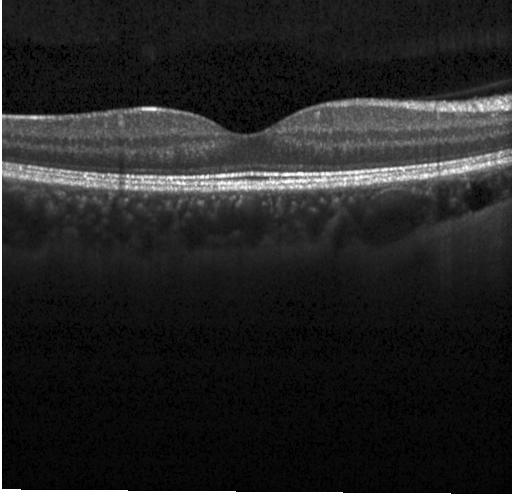 Through the macula. SD-OCT. Instrument: Heidelberg Spectralis. OCT B-scan.
Macular OCT: no evidence of choroidal neovascularization, diabetic macular edema, or drusen.